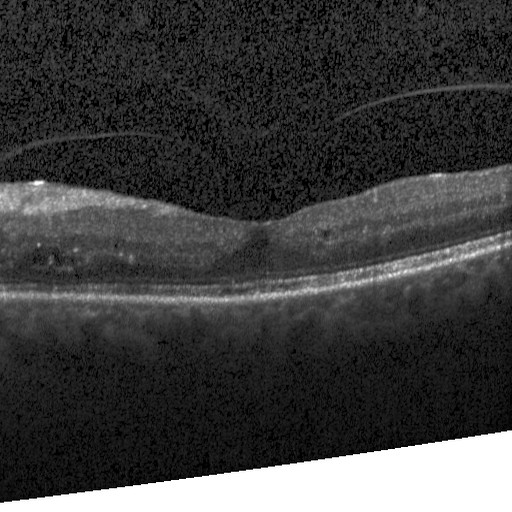
OCT finding: diabetic macular edema.